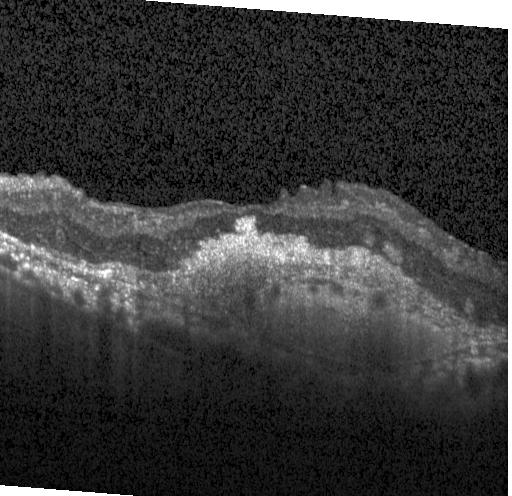

Spectral-domain OCT, retinal OCT cross-section.
Assessment: CNV.